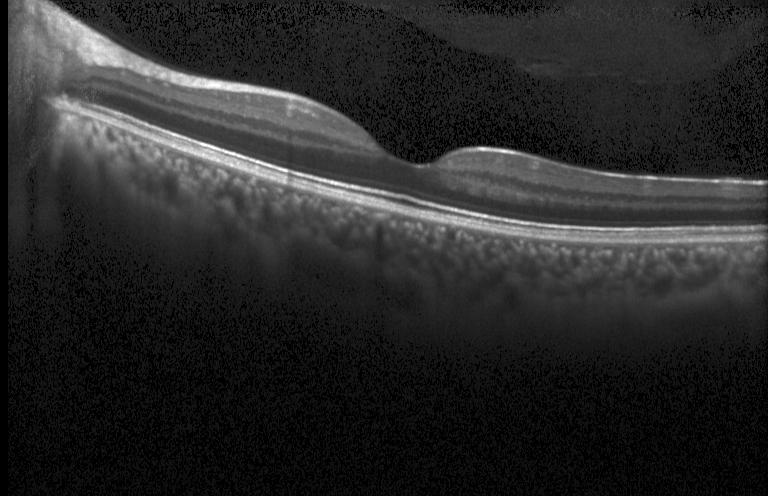
Acquired on a Heidelberg Spectralis, SD-OCT, horizontal scan through the fovea, optical coherence tomography scan.
The scan shows no choroidal neovascularization, no diabetic macular edema, and no drusen.